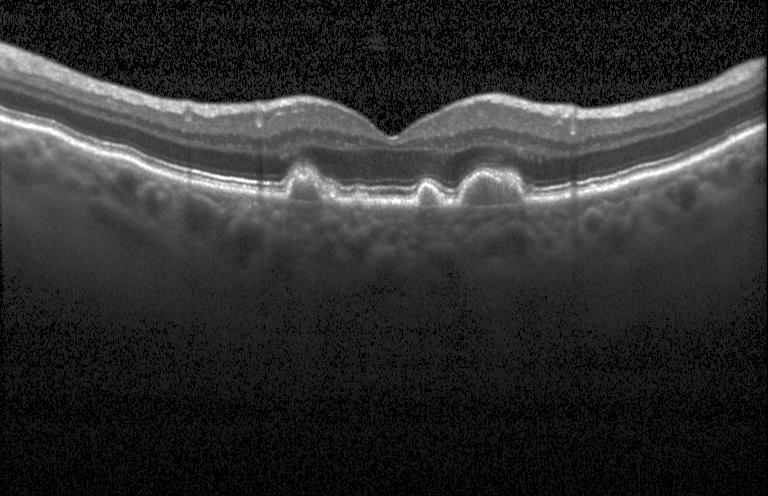

OCT B-scan showing drusen.